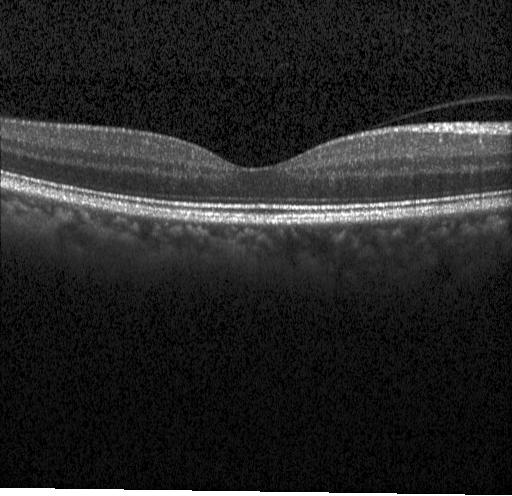

OCT finding: no choroidal neovascularization, no diabetic macular edema, and no drusen.